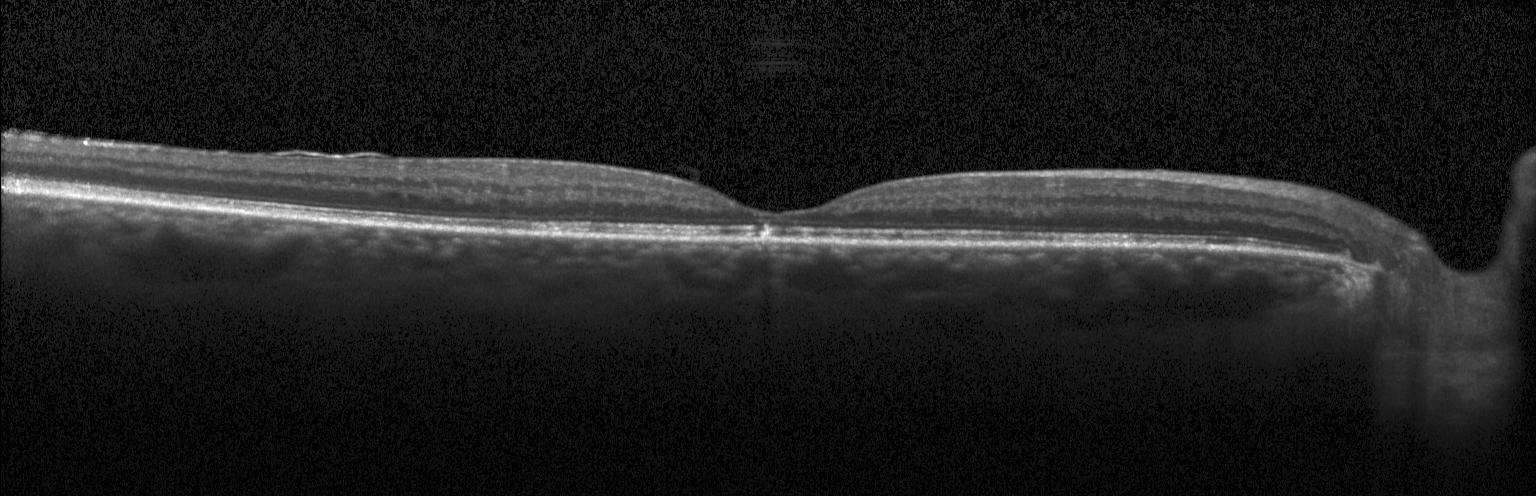 Instrument: Heidelberg Spectralis, centered on the fovea, SD-OCT, OCT line scan. Finding: no evidence of choroidal neovascularization, diabetic macular edema, or drusen.